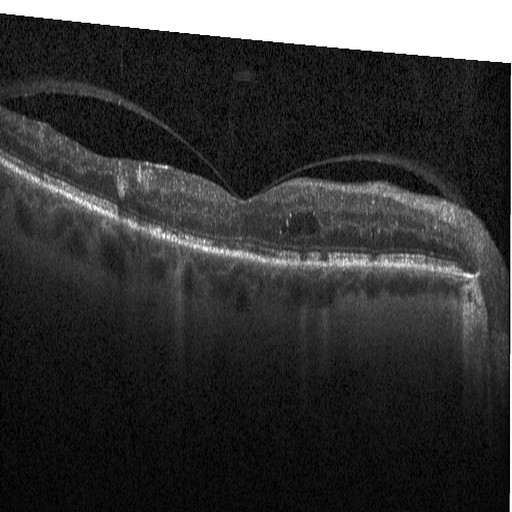 Macular OCT: diabetic macular edema.